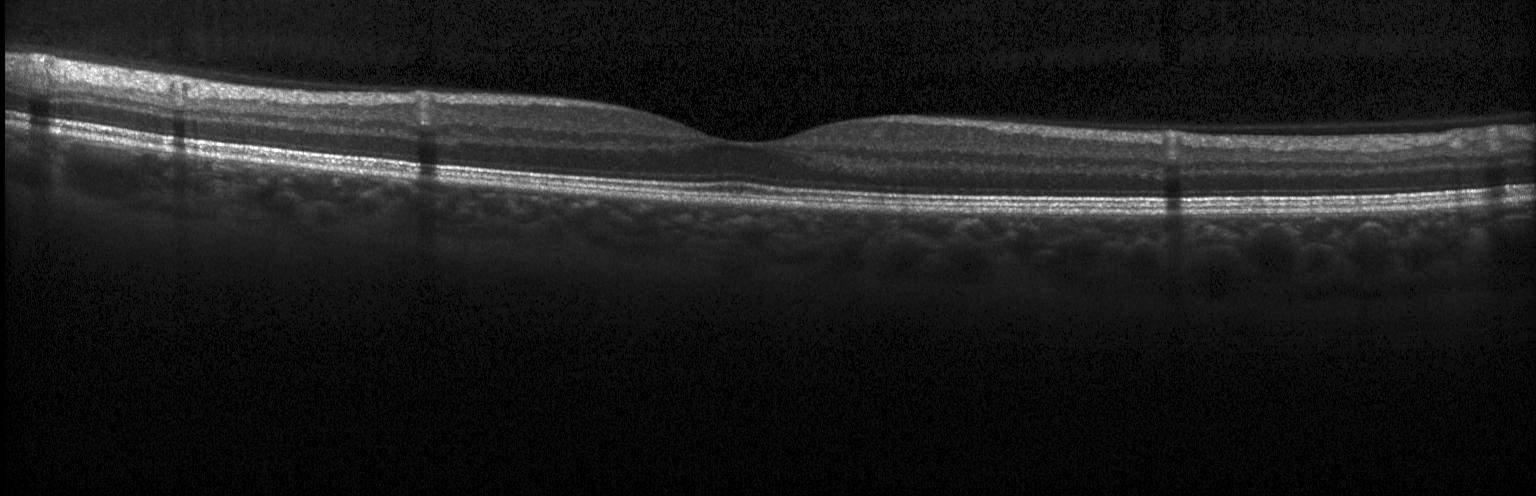 Impression: no choroidal neovascularization, no diabetic macular edema, and no drusen.